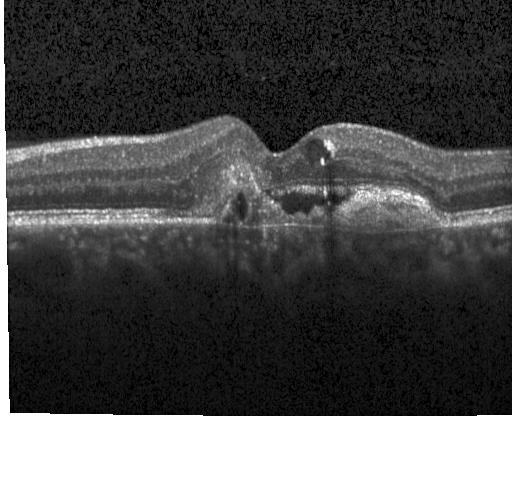 A choroidal neovascular membrane.